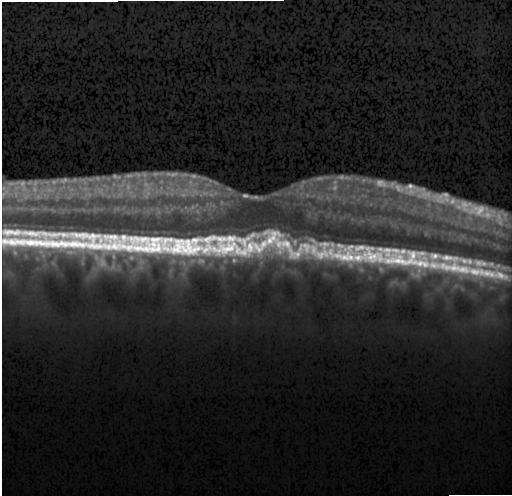 Centered on the fovea, retinal OCT cross-section.
Drusen.